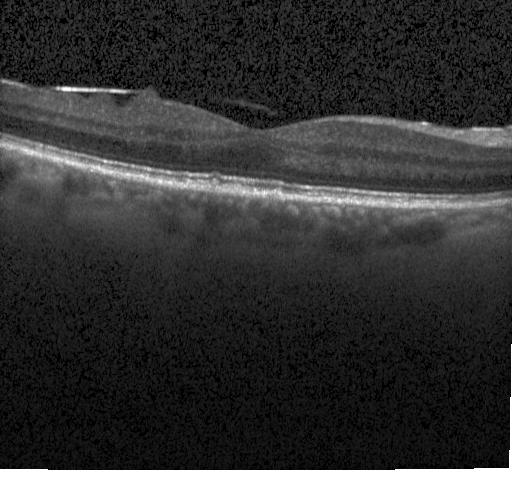 Heidelberg Spectralis OCT system · optical coherence tomography scan · spectral-domain OCT. Finding: sub-RPE drusenoid deposits.